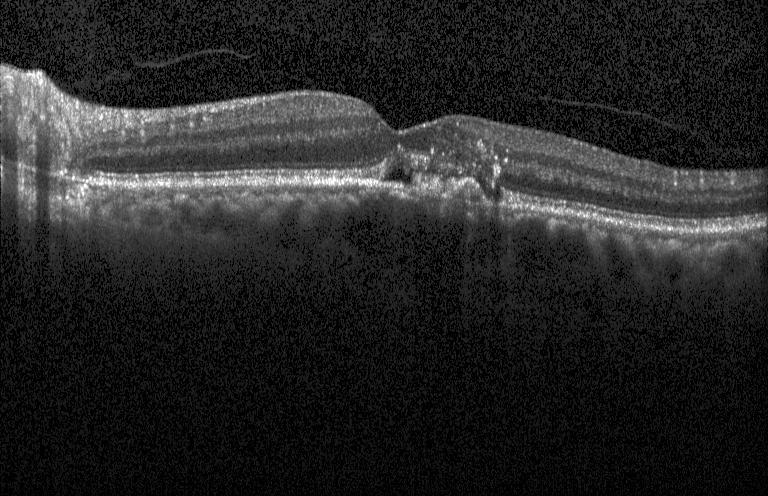

Instrument: Heidelberg Spectralis · SD-OCT · OCT B-scan · fovea-centered — Impression: CNV.